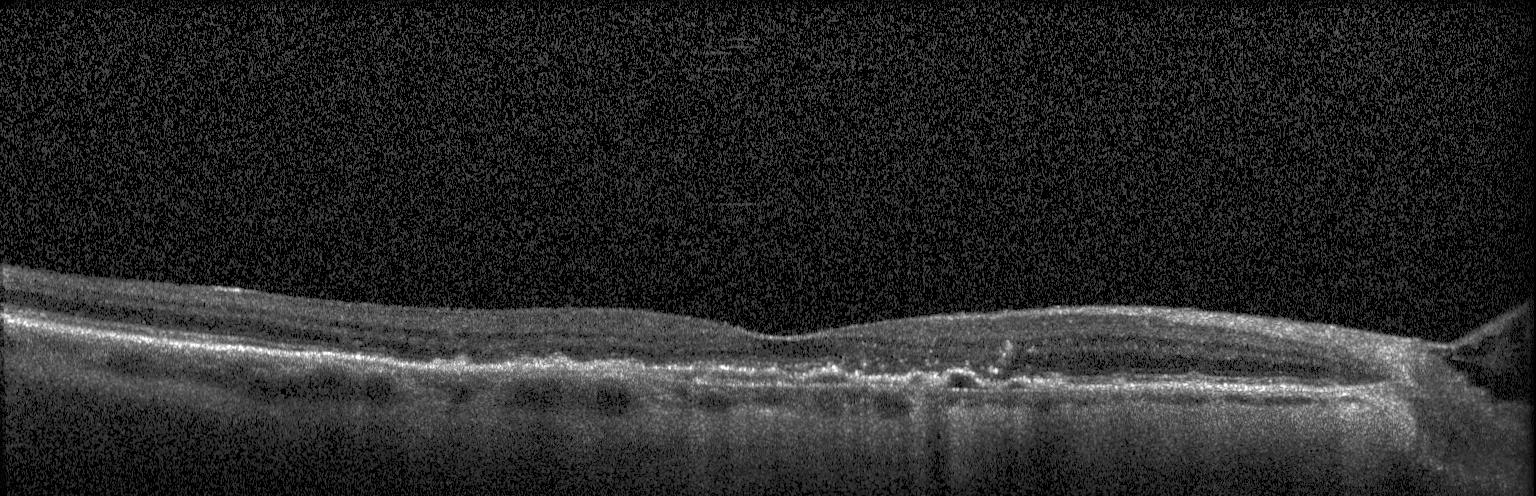

Retinal OCT B-scan · macular scan — This B-scan demonstrates a choroidal neovascular membrane.